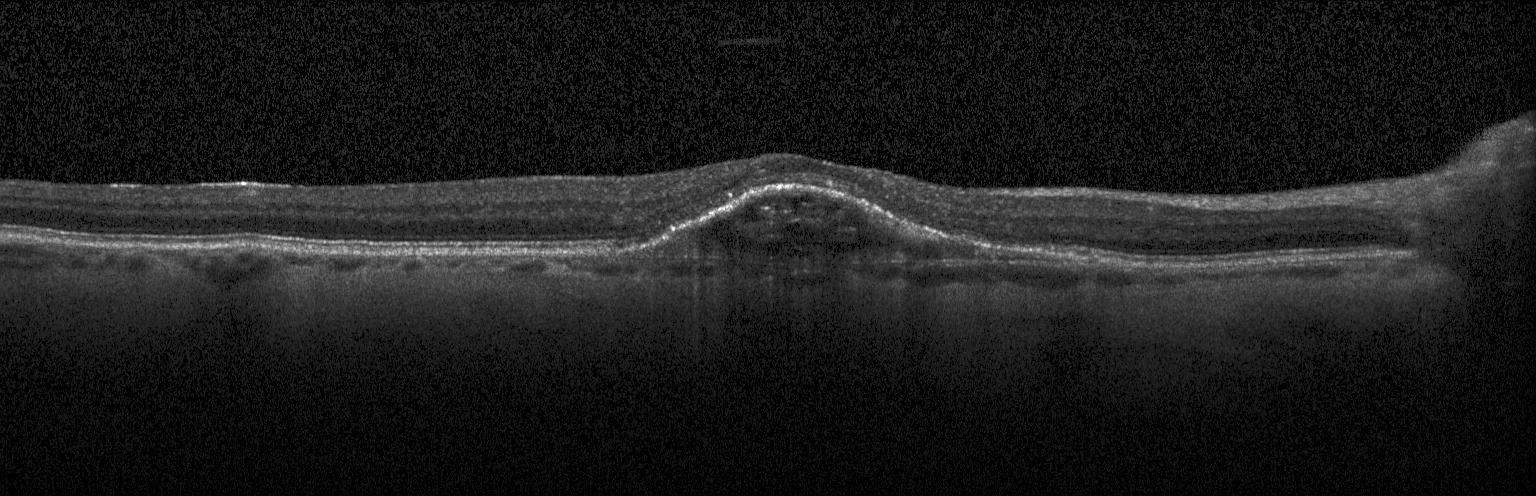

OCT B-scan.
Impression: CNV.